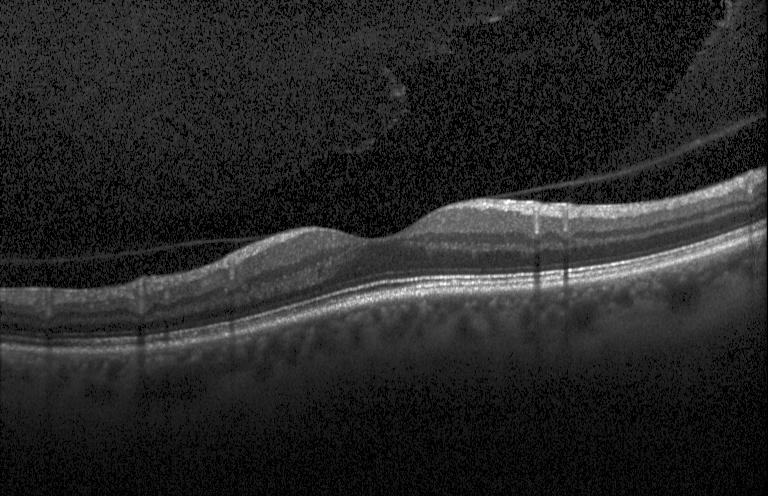

The scan shows no evidence of CNV, DME, or drusen.